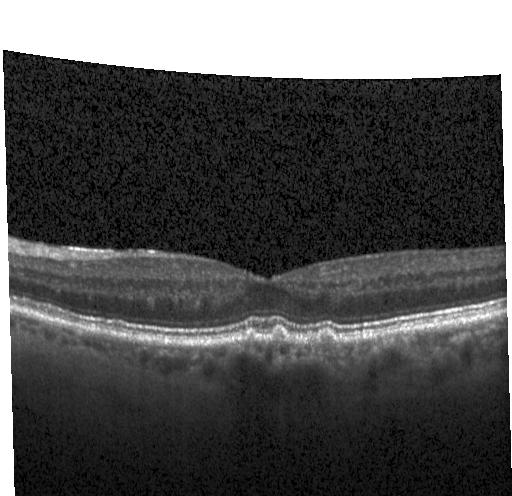

Dx: drusen.